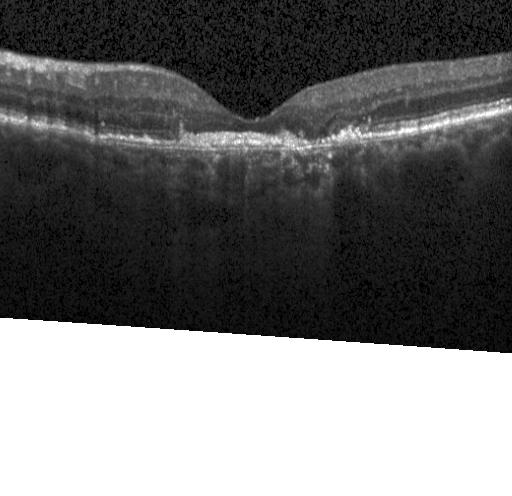

Through the macula, retinal OCT B-scan, spectral-domain OCT.
Diagnosis: a choroidal neovascular membrane.